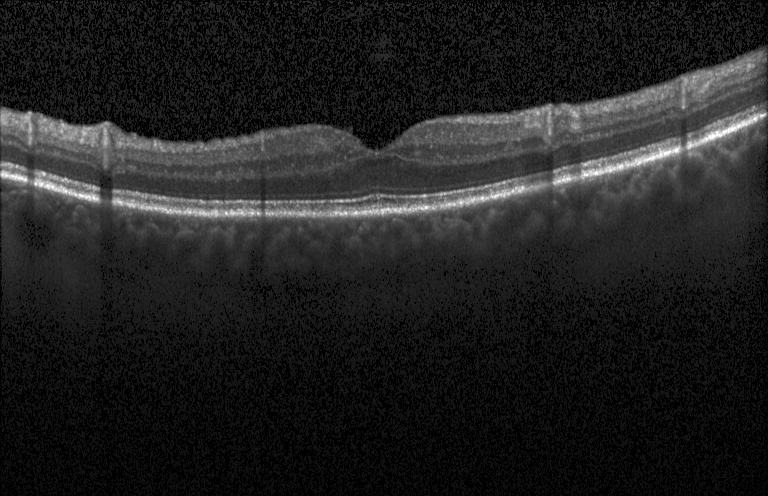 Finding: no CNV, no DME, and no drusen.